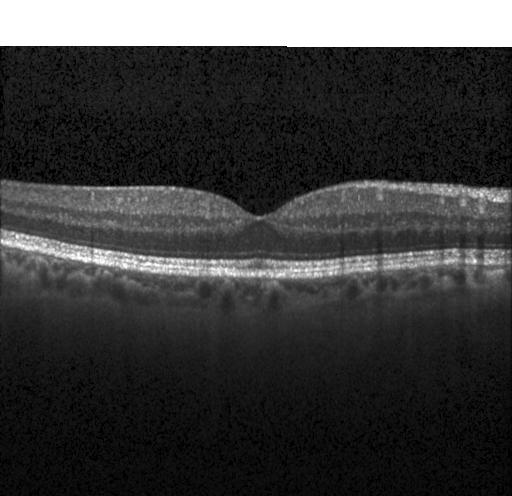
Macular OCT demonstrating no evidence of choroidal neovascularization, diabetic macular edema, or drusen.